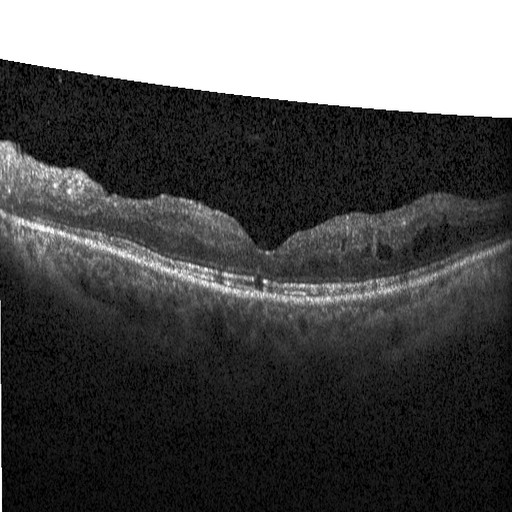 This B-scan demonstrates diabetic macular edema.